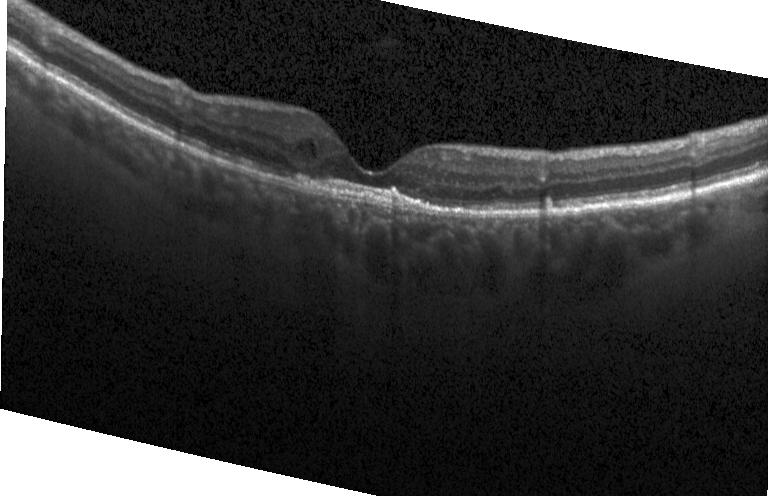 Assessment: a choroidal neovascular membrane.